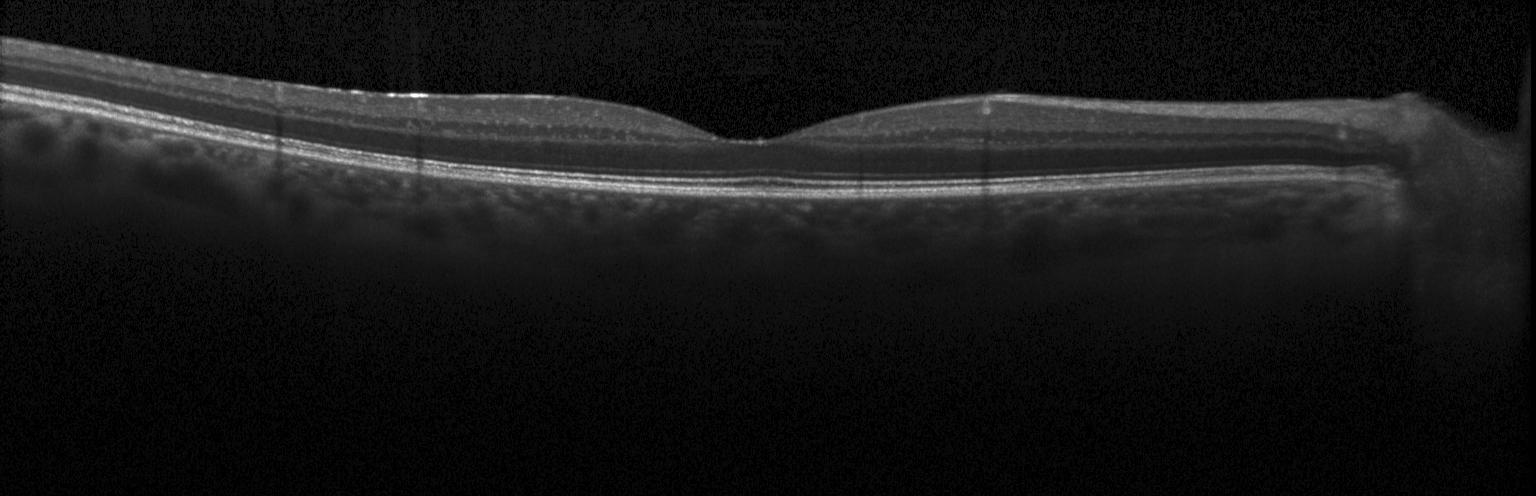

Macular OCT: no evidence of choroidal neovascularization, diabetic macular edema, or drusen.